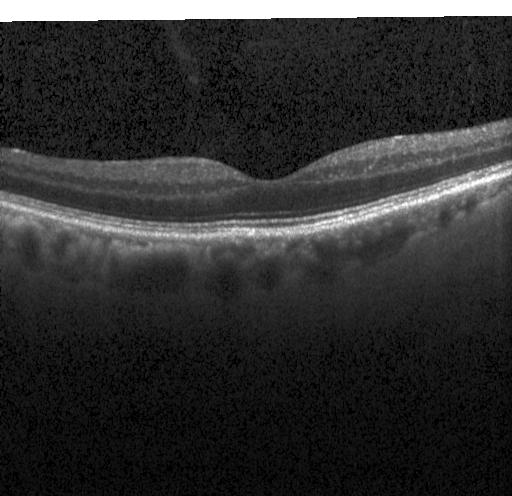 Impression: no evidence of CNV, DME, or drusen.